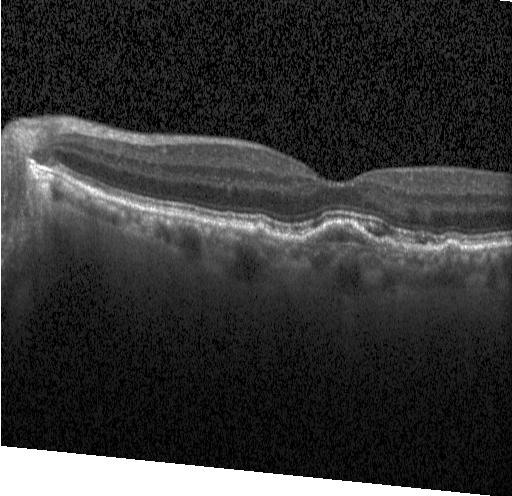 Spectral-domain optical coherence tomography. Optical coherence tomography scan. Through the macula. Heidelberg Spectralis.
Finding: a choroidal neovascular membrane.